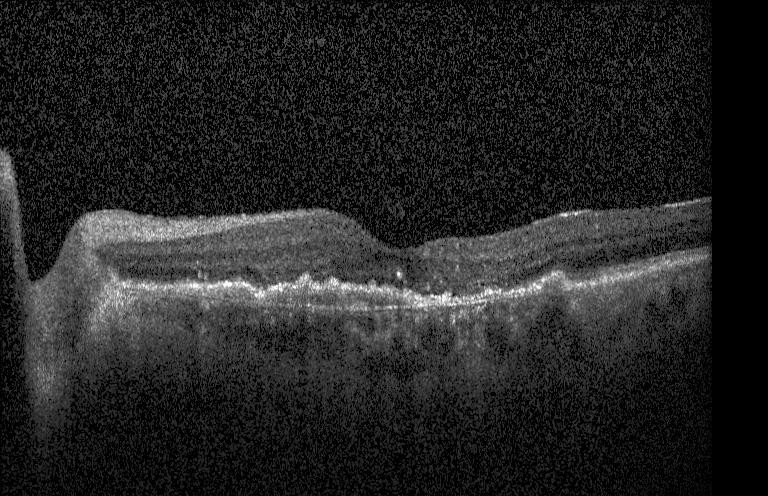
Assessment: choroidal neovascularization.